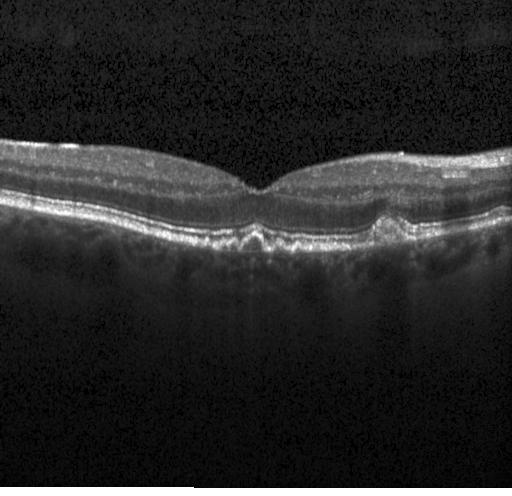 Retinal OCT B-scan; horizontal scan through the fovea.
Diagnosis: choroidal neovascularization (CNV).